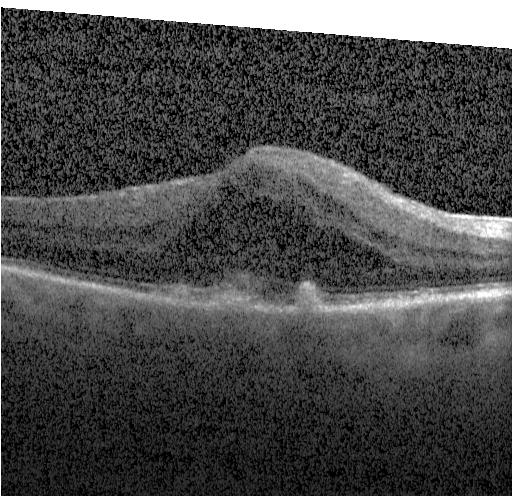
Heidelberg Spectralis, retinal OCT cross-section, fovea-centered — Impression: choroidal neovascularization (CNV).